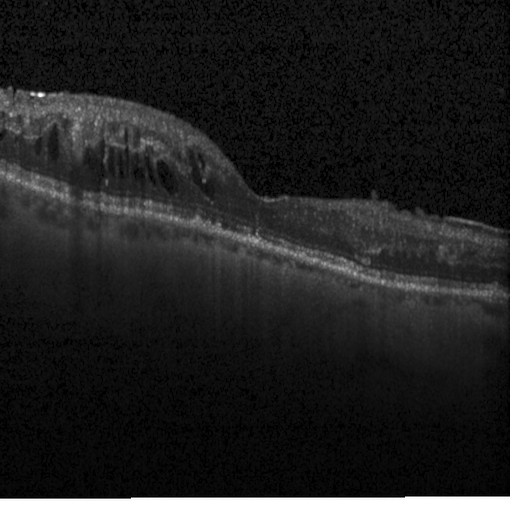 Optical coherence tomography B-scan, SD-OCT, Heidelberg Spectralis OCT system, horizontal scan through the fovea. The scan shows DME.